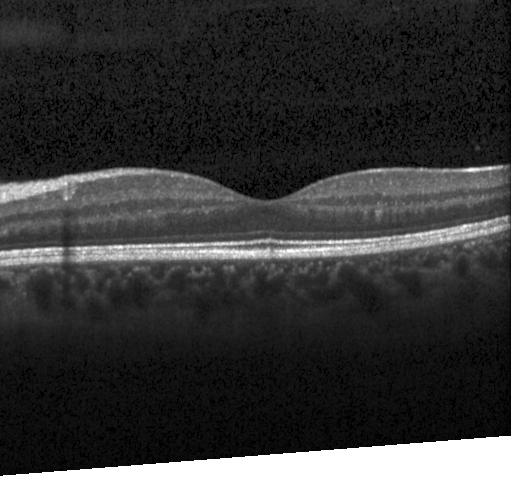

Instrument: Heidelberg Spectralis, horizontal scan through the fovea, optical coherence tomography scan
OCT finding: no evidence of choroidal neovascularization, diabetic macular edema, or drusen.